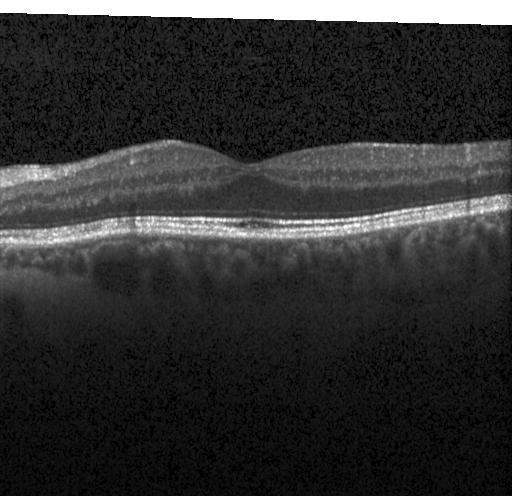
Macular OCT: no choroidal neovascularization, diabetic macular edema, or drusen.